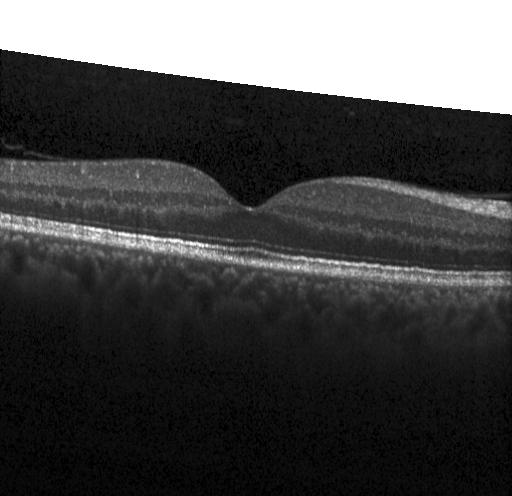 Assessment: no choroidal neovascularization, diabetic macular edema, or drusen.